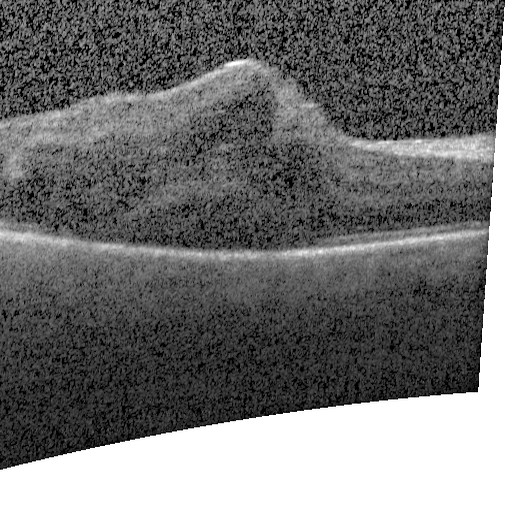

Instrument: Heidelberg Spectralis. Optical coherence tomography scan. Spectral-domain optical coherence tomography. Through the macula.
Impression: DME.